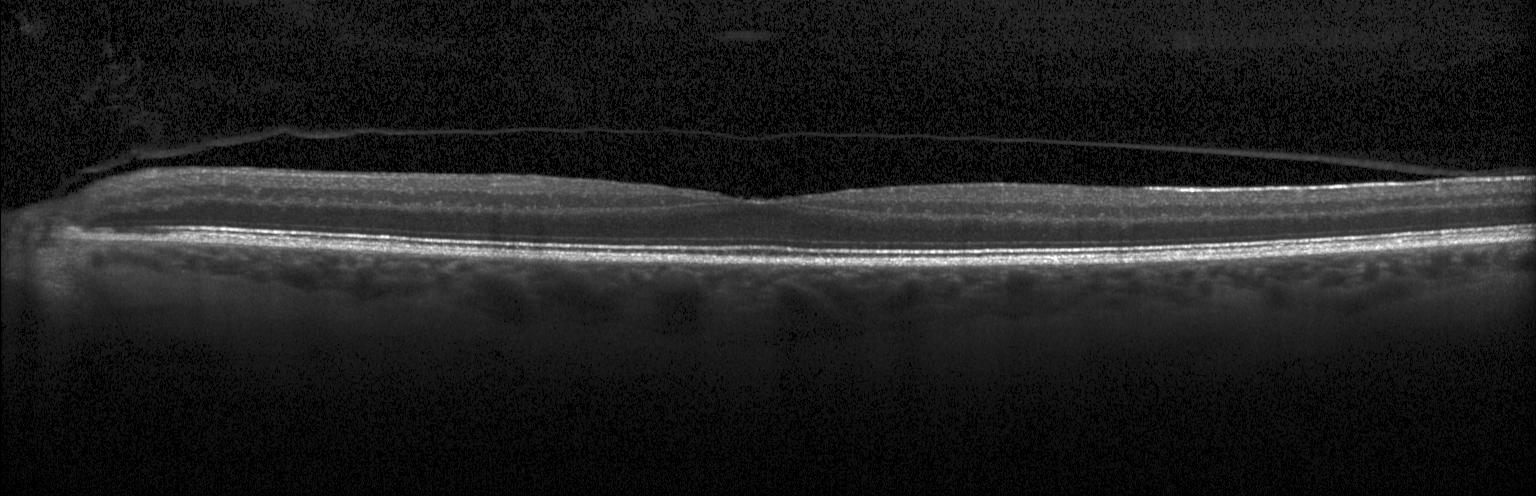
Optical coherence tomography scan; macular scan; Heidelberg Spectralis OCT system; spectral-domain OCT — Impression: no CNV, DME, or drusen.